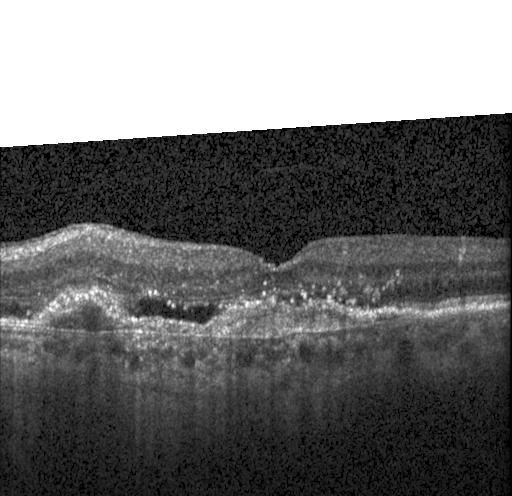
Spectral-domain optical coherence tomography, OCT line scan. Assessment: CNV.